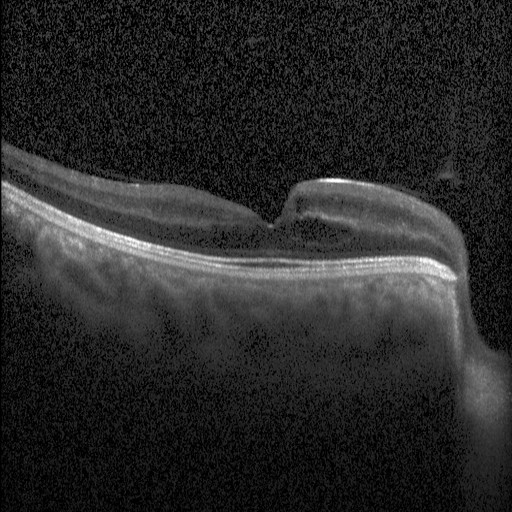
Instrument: Heidelberg Spectralis. Spectral-domain OCT. Centered on the fovea. OCT line scan. Macular OCT: diabetic macular edema.